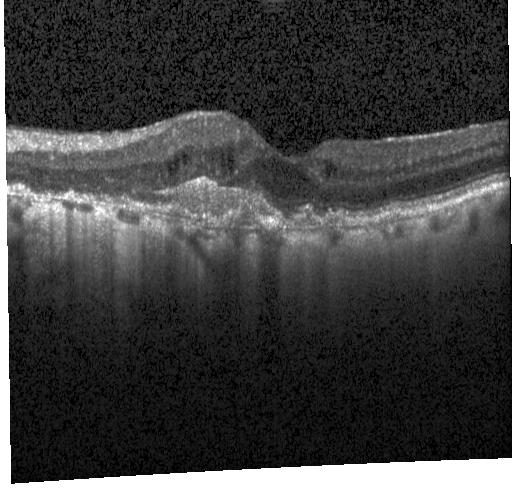

OCT line scan — A choroidal neovascular membrane.